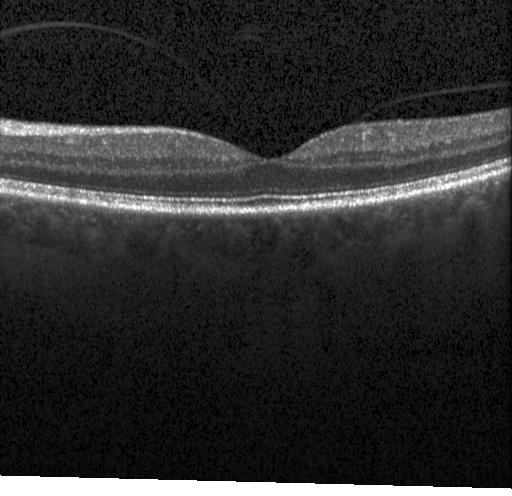
Diagnosis: no choroidal neovascularization, diabetic macular edema, or drusen.